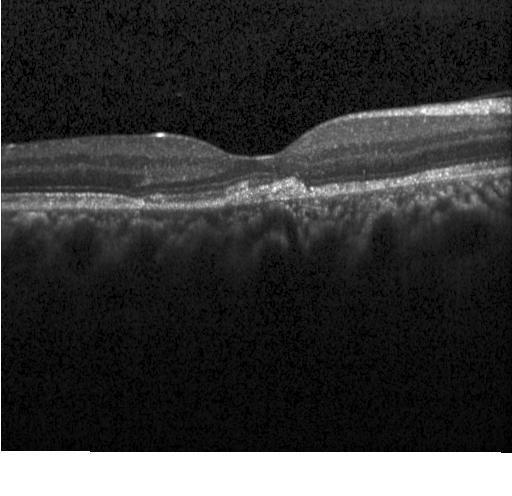 OCT scan showing CNV.